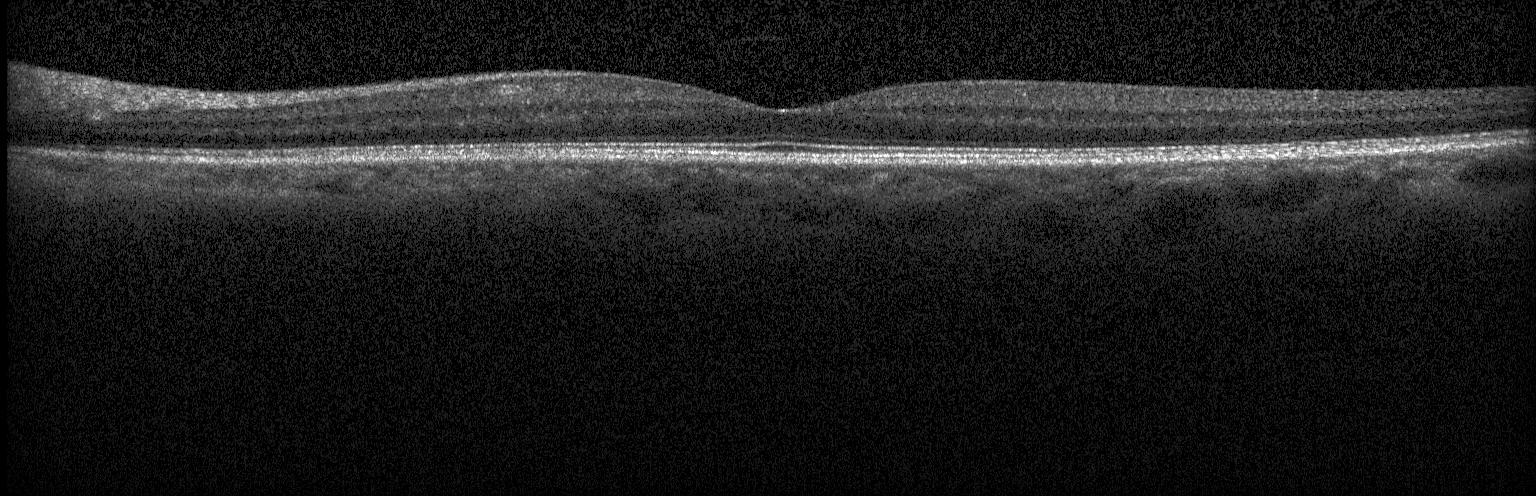 Finding: no evidence of CNV, DME, or drusen.